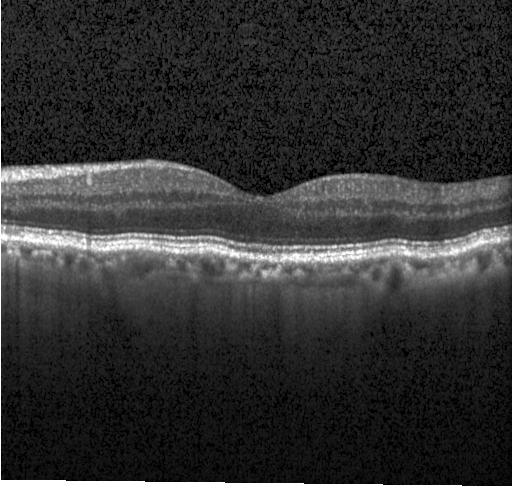
Optical coherence tomography scan. Centered on the fovea — Impression: no CNV, no DME, and no drusen.